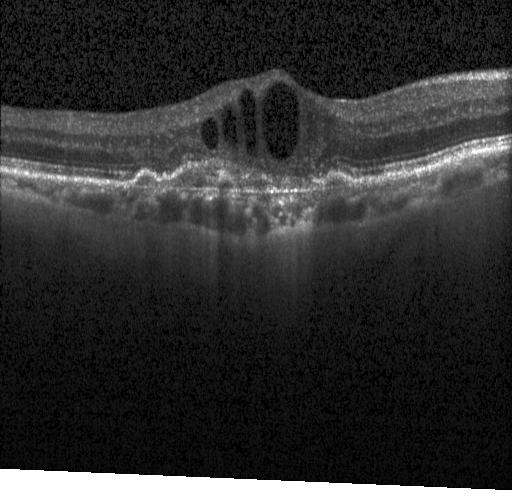 Retinal OCT cross-section. Macular OCT: CNV.